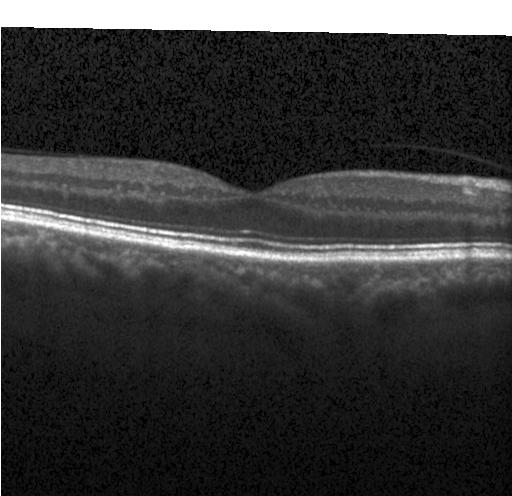
Optical coherence tomography B-scan; spectral-domain optical coherence tomography.
Macular OCT: no choroidal neovascularization, no diabetic macular edema, and no drusen.